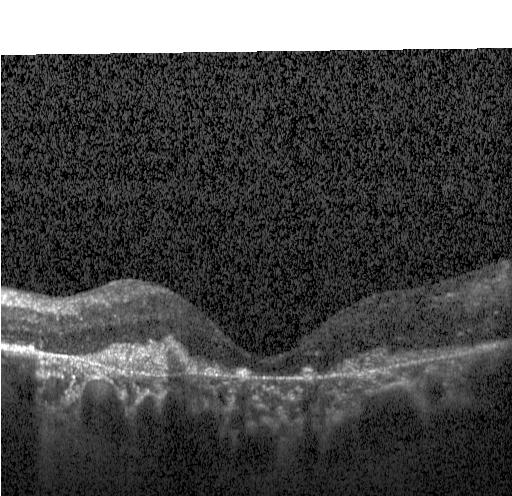
Diagnosis: a choroidal neovascular membrane.